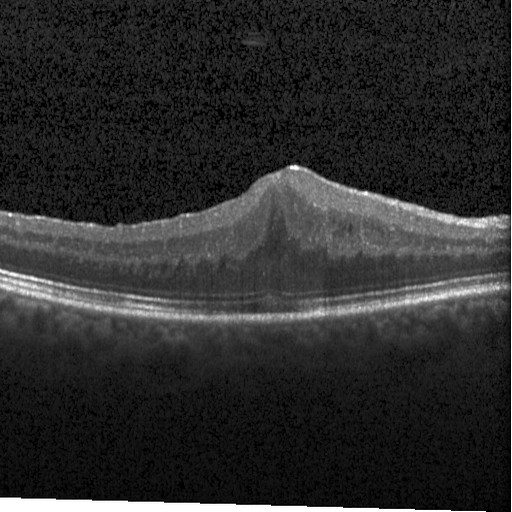
Retinal OCT cross-section, macular scan, instrument: Heidelberg Spectralis.
Diabetic macular edema.